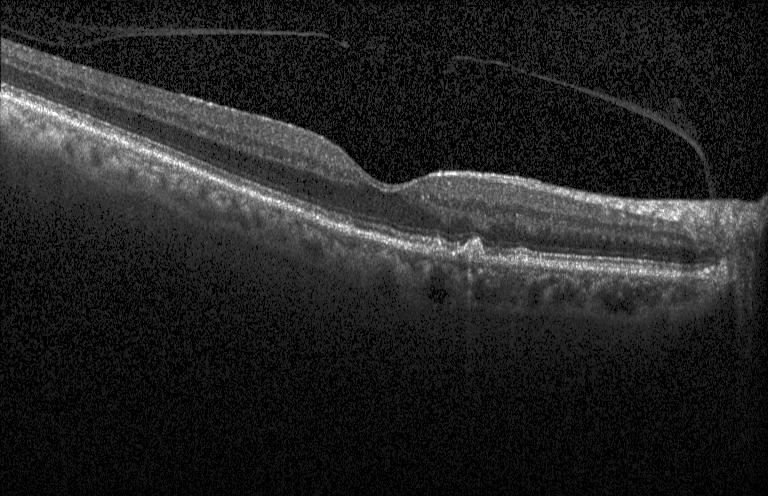

OCT scan showing drusen.